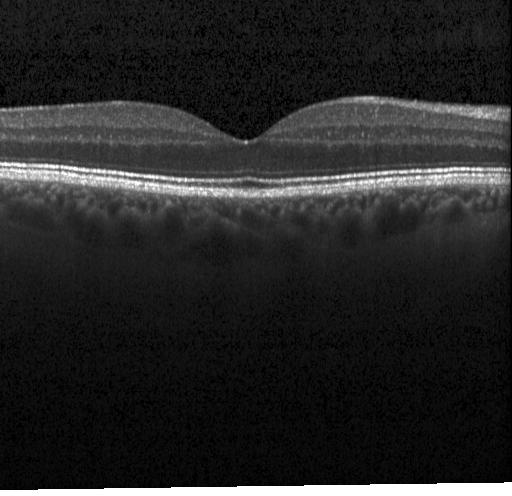

Macular OCT: no evidence of choroidal neovascularization, diabetic macular edema, or drusen.